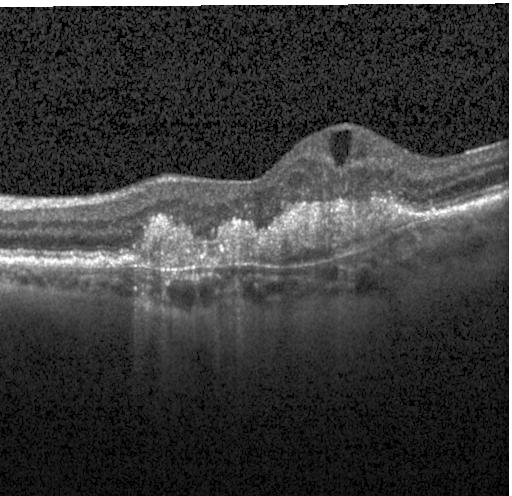
Spectral-domain OCT. Optical coherence tomography scan. Instrument: Heidelberg Spectralis. Impression: CNV.